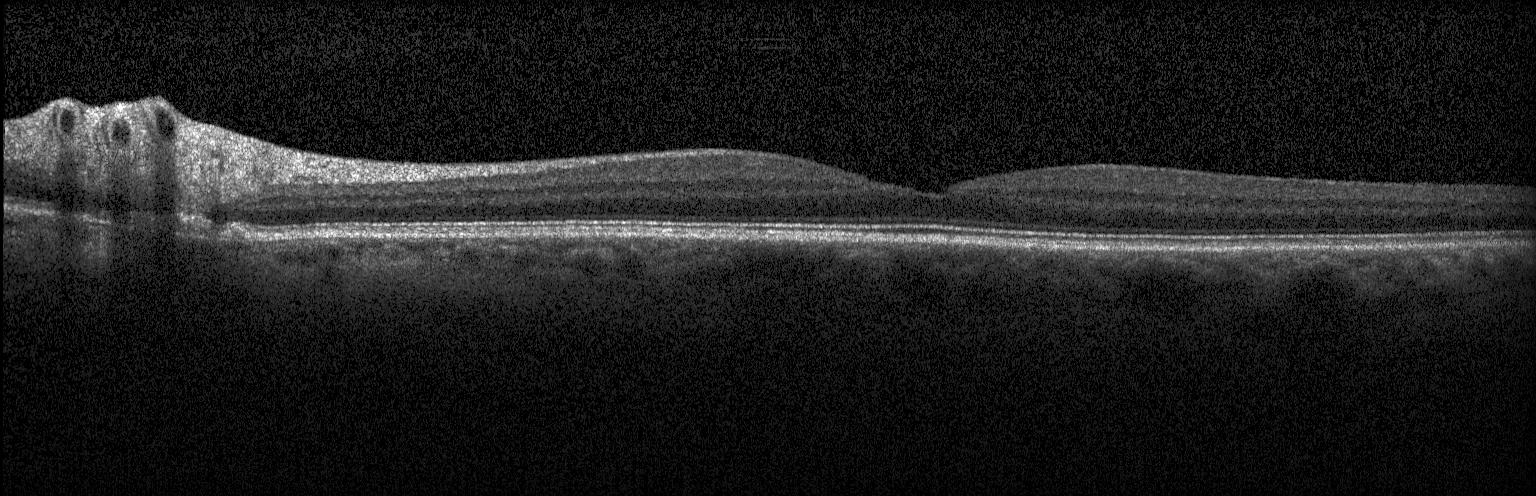

Retinal OCT cross-section · SD-OCT · acquired on a Heidelberg Spectralis.
Diagnosis: no choroidal neovascularization, no diabetic macular edema, and no drusen.